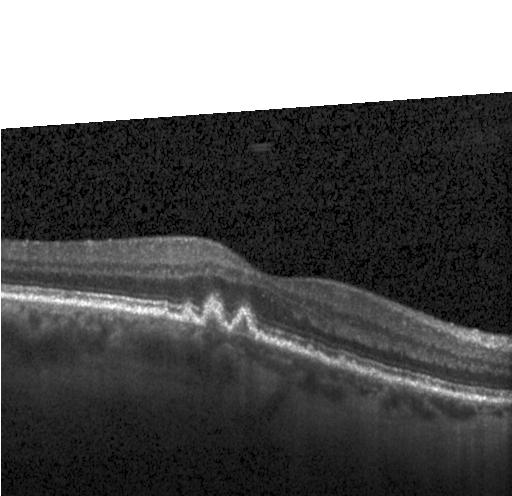
OCT B-scan; fovea-centered. Impression: multiple drusen.